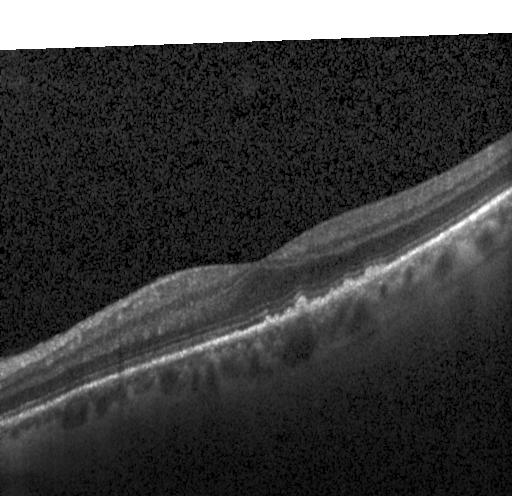
Retinal OCT cross-section showing drusen.